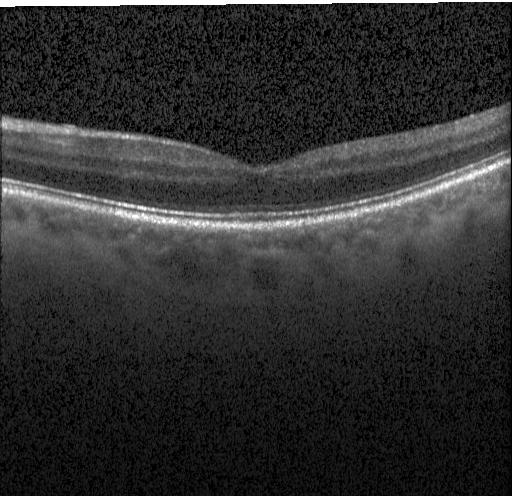
Horizontal scan through the fovea; instrument: Heidelberg Spectralis; optical coherence tomography B-scan; spectral-domain OCT.
OCT finding: no choroidal neovascularization, diabetic macular edema, or drusen.